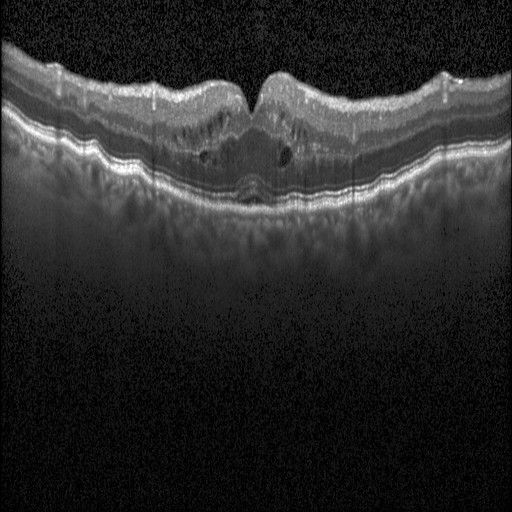
DME.